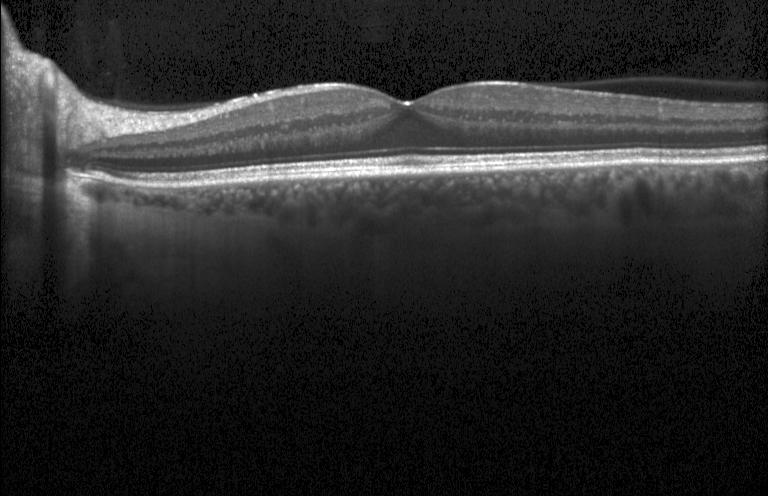

Through the macula · spectral-domain optical coherence tomography · optical coherence tomography B-scan.
No CNV, DME, or drusen.